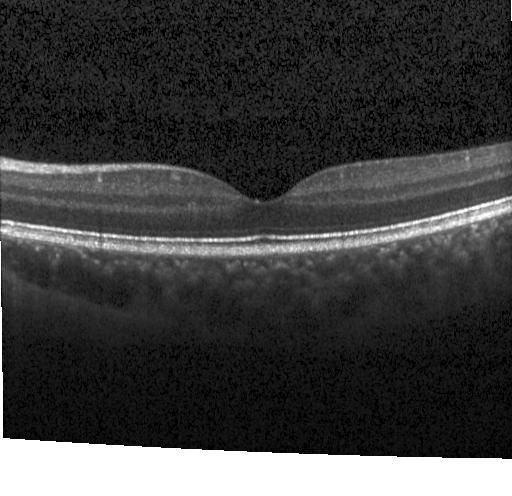 Retinal OCT cross-section — Finding: no choroidal neovascularization, diabetic macular edema, or drusen.